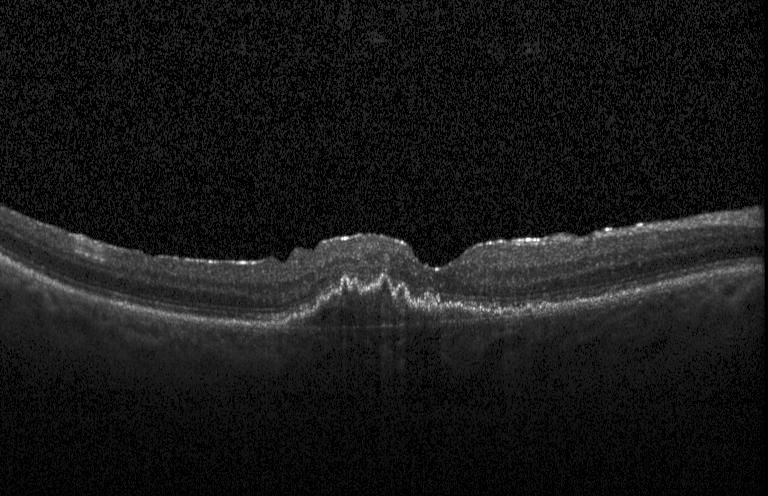

Spectral-domain optical coherence tomography · Heidelberg Spectralis · OCT line scan.
Macular OCT: a choroidal neovascular membrane.